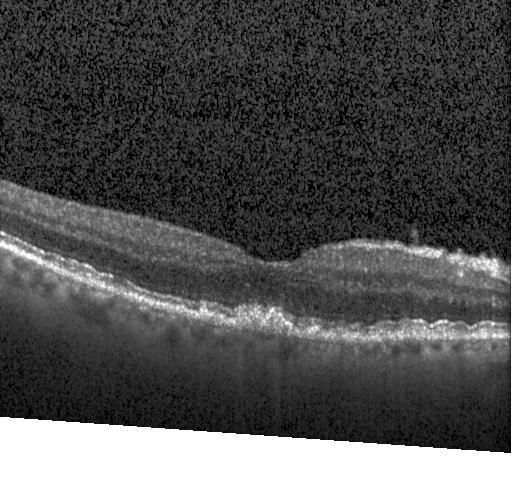

Spectral-domain OCT. OCT line scan. Centered on the fovea
Diagnosis: multiple drusen.